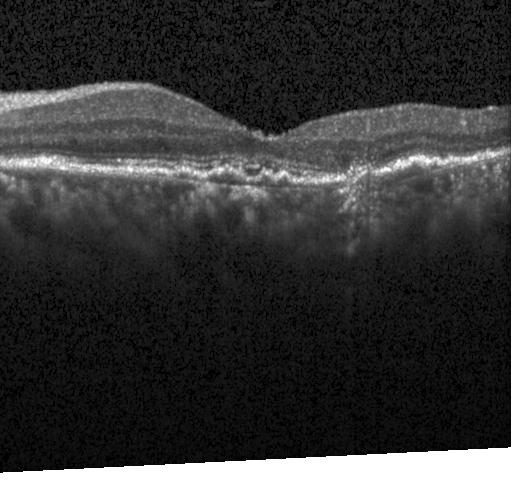 Assessment: CNV.